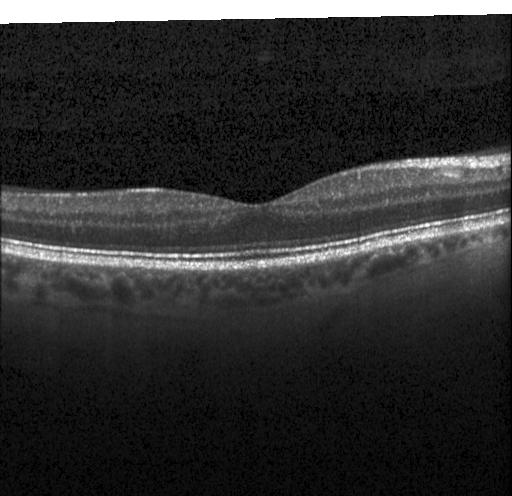

Assessment: neither choroidal neovascularization, diabetic macular edema, nor drusen.